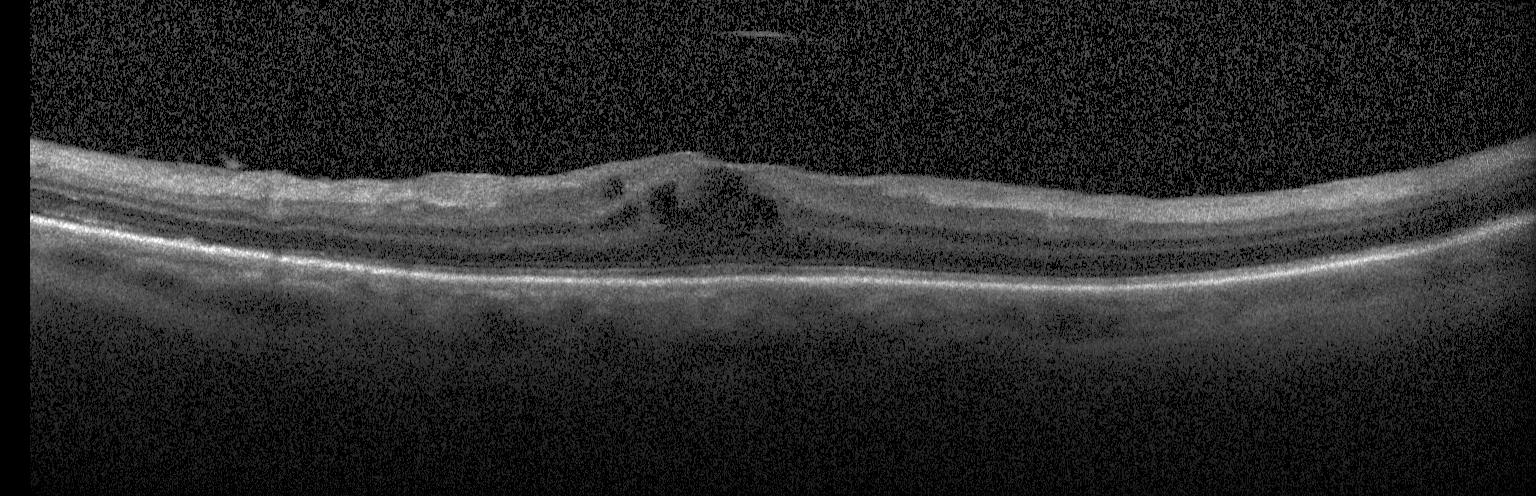 Spectral-domain optical coherence tomography. Retinal OCT B-scan — Assessment: DME.